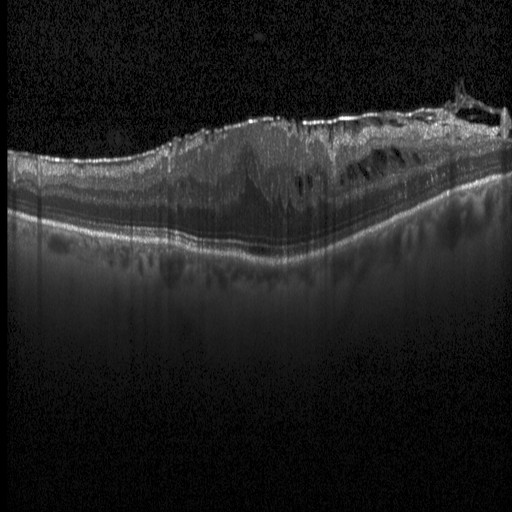

Impression: diabetic macular edema.